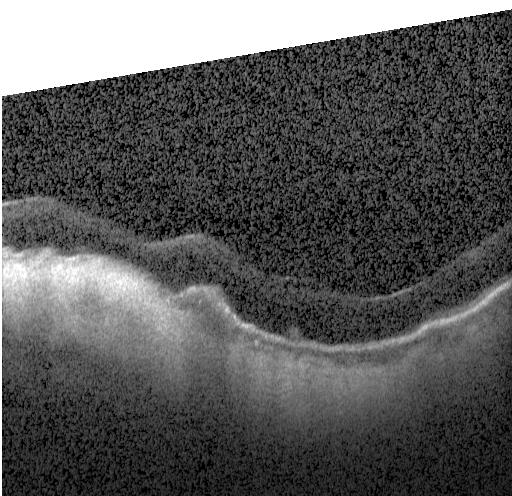

Macular OCT demonstrating a choroidal neovascular membrane.